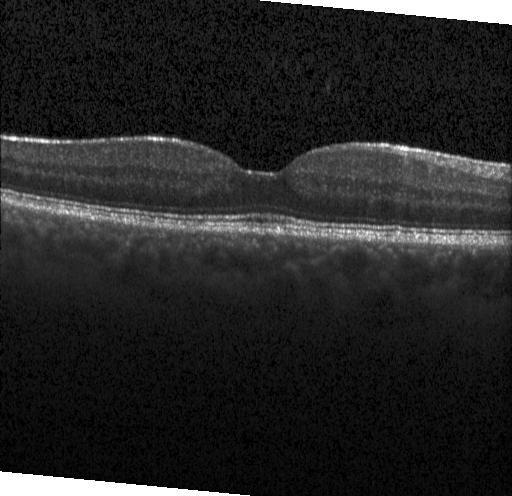

Diagnosis: no choroidal neovascularization, diabetic macular edema, or drusen.